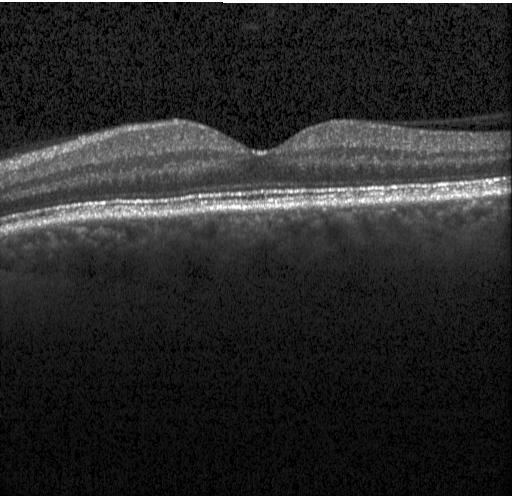

Macular scan · optical coherence tomography scan. Finding: no choroidal neovascularization, no diabetic macular edema, and no drusen.